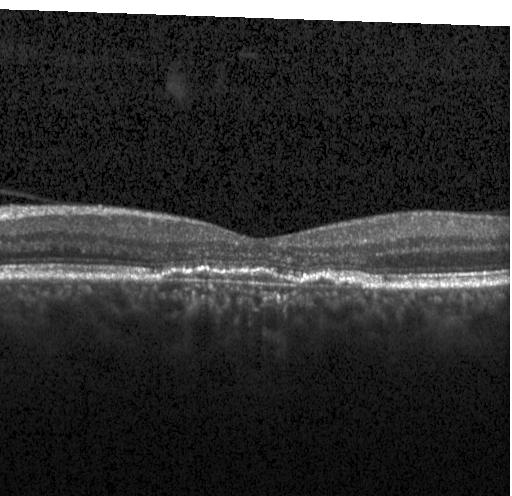

Retinal OCT B-scan. A choroidal neovascular membrane.